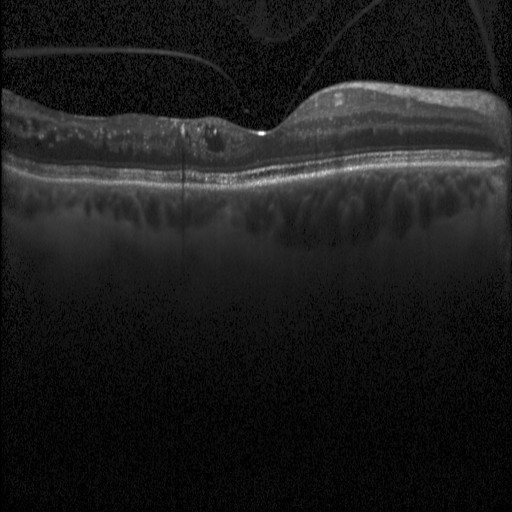 Spectral-domain optical coherence tomography; retinal OCT cross-section — Impression: DME.